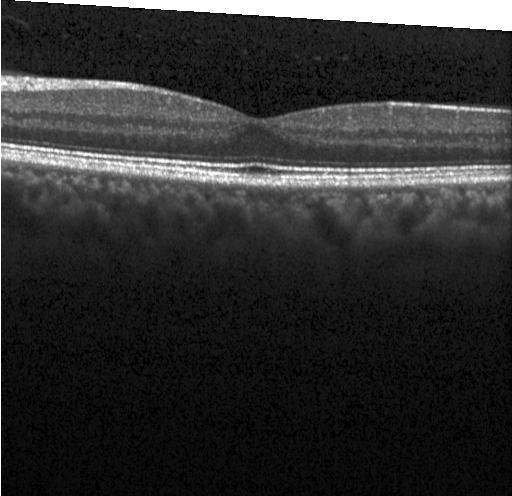

Horizontal scan through the fovea, OCT B-scan.
Diagnosis: no choroidal neovascularization, no diabetic macular edema, and no drusen.